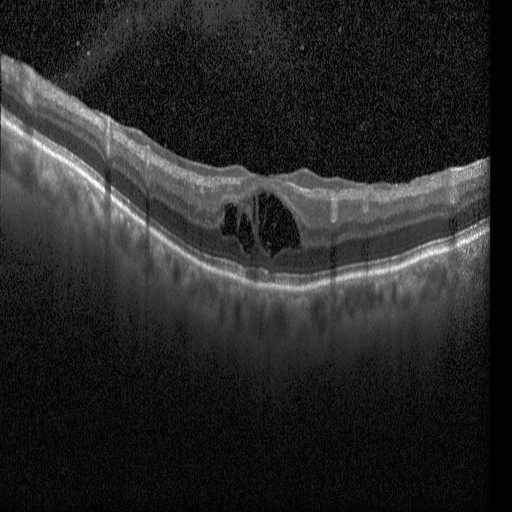
Acquired on a Heidelberg Spectralis, OCT B-scan. Impression: diabetic macular edema (DME).